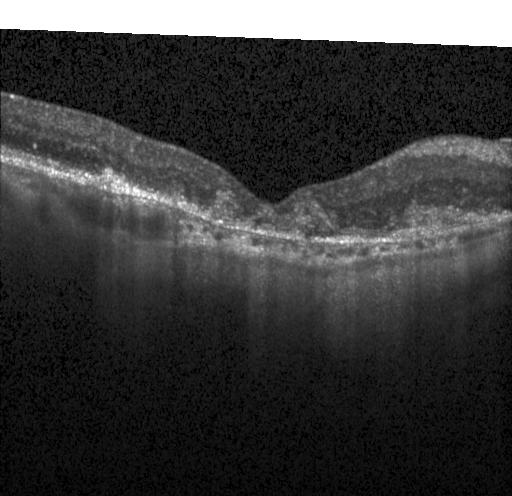

Heidelberg Spectralis; retinal OCT cross-section; spectral-domain optical coherence tomography; centered on the fovea
Finding: choroidal neovascularization (CNV).